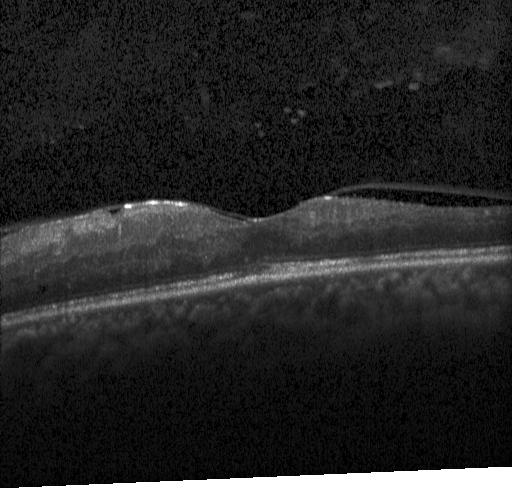
The scan shows diabetic macular edema.